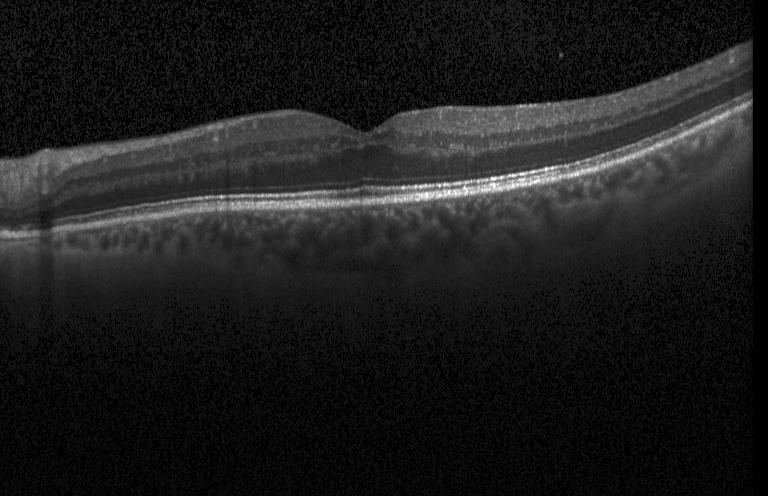
Retinal OCT B-scan.
Assessment: no choroidal neovascularization, no diabetic macular edema, and no drusen.